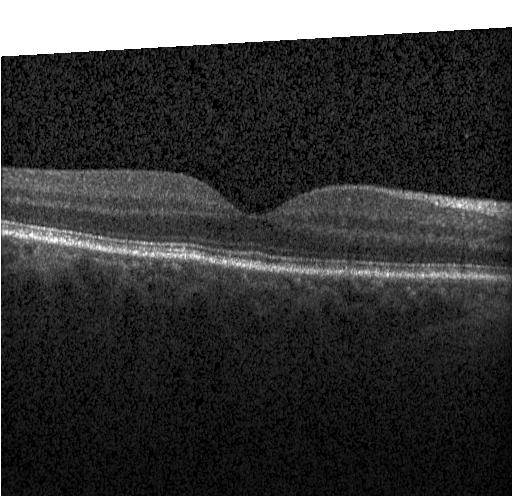 No choroidal neovascularization, no diabetic macular edema, and no drusen.